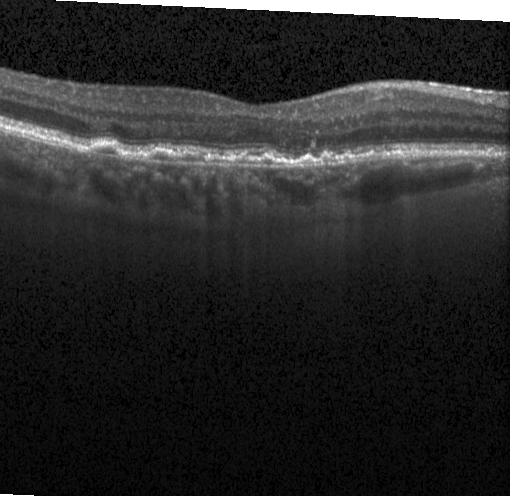
OCT line scan, through the macula, Heidelberg Spectralis, spectral-domain optical coherence tomography.
Macular OCT: a choroidal neovascular membrane.